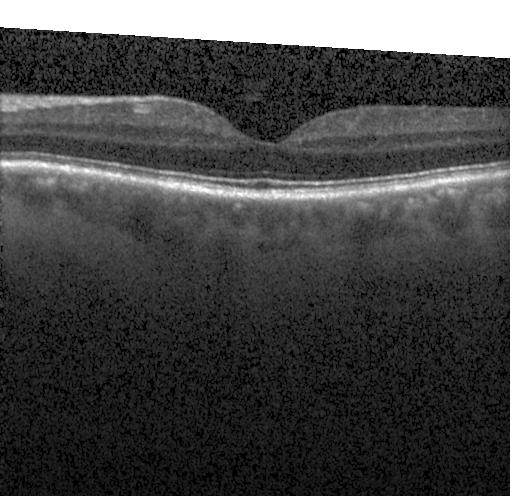 Diagnosis: no CNV, DME, or drusen.